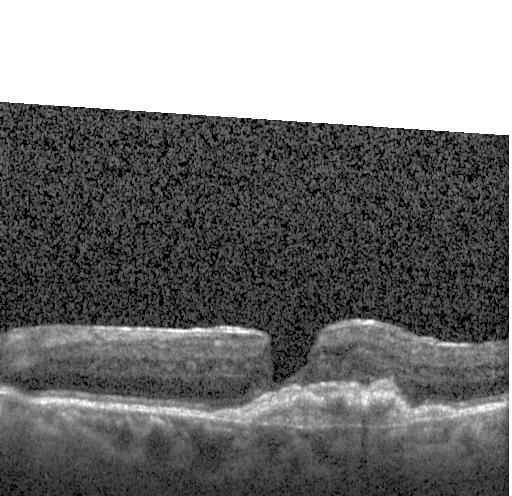

OCT line scan. Horizontal scan through the fovea. Heidelberg Spectralis OCT system. SD-OCT — OCT finding: a choroidal neovascular membrane.